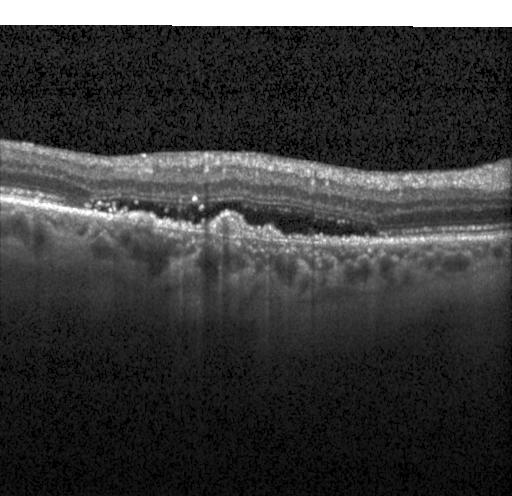 Through the macula · Heidelberg Spectralis · optical coherence tomography scan. OCT finding: a choroidal neovascular membrane.